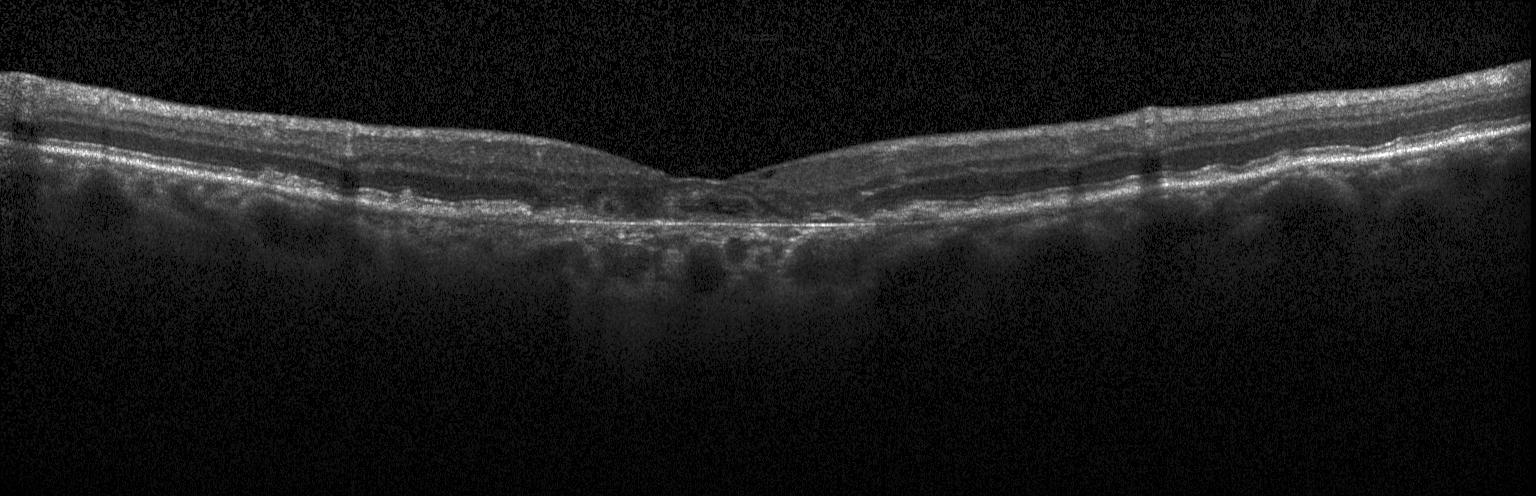
This B-scan demonstrates choroidal neovascularization.